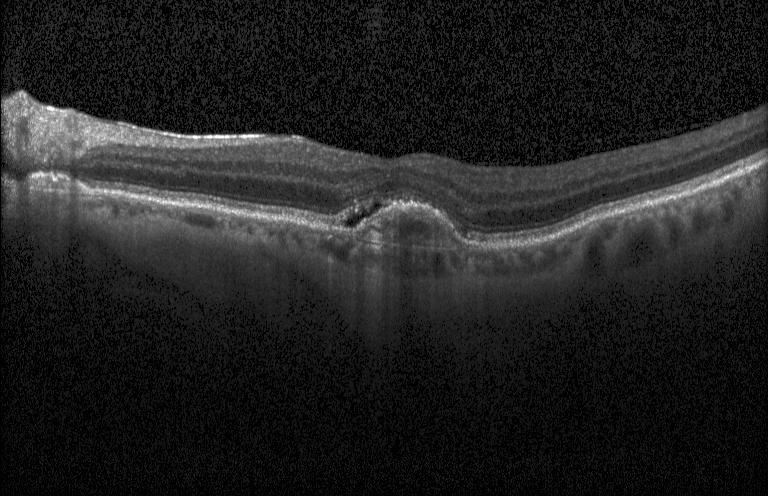

OCT scan showing CNV.